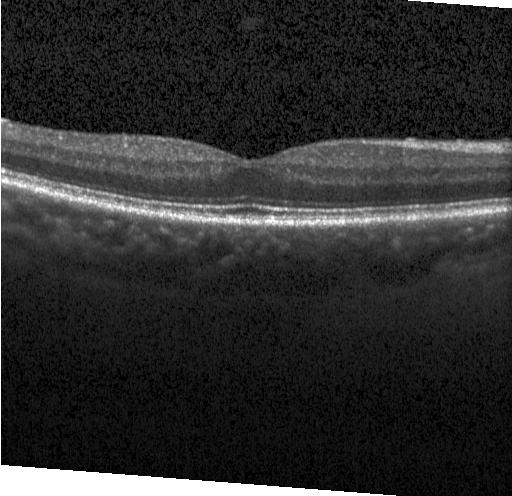 OCT B-scan
Finding: no evidence of choroidal neovascularization, diabetic macular edema, or drusen.